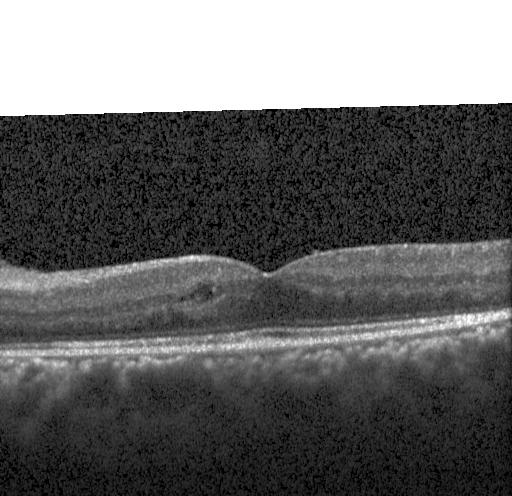

OCT finding: diabetic macular edema (DME).